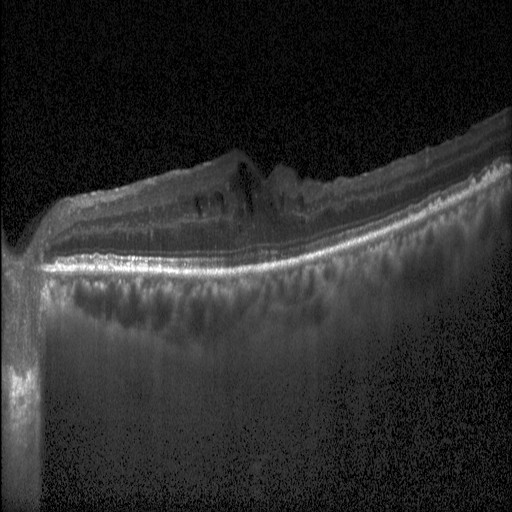
OCT scan showing diabetic macular edema (DME).